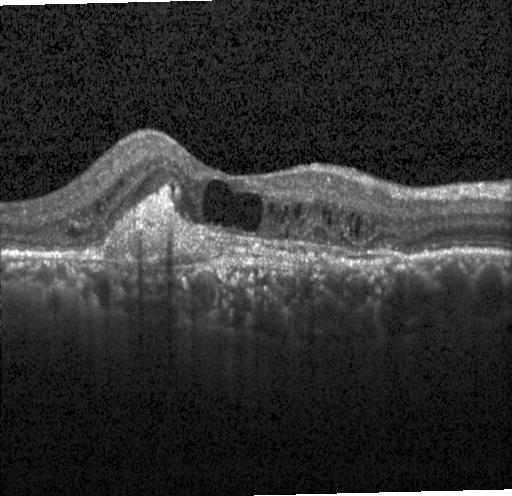

Acquired on a Heidelberg Spectralis, OCT B-scan, SD-OCT, centered on the fovea.
Diagnosis: choroidal neovascularization (CNV).